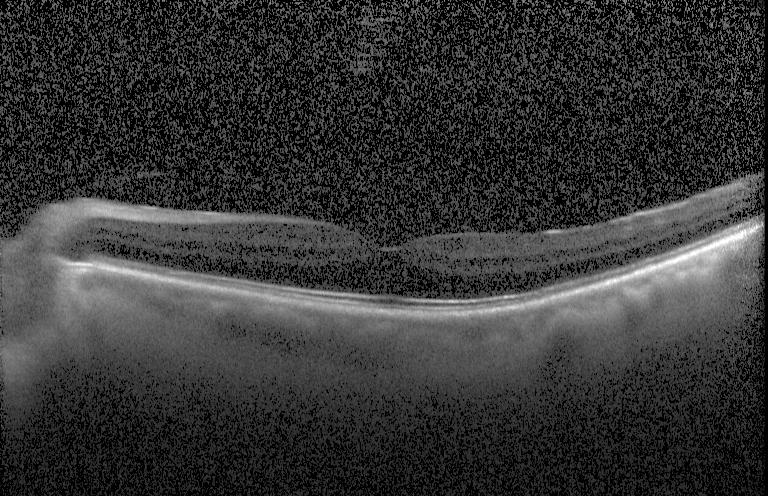
Optical coherence tomography B-scan — Neither choroidal neovascularization, diabetic macular edema, nor drusen.